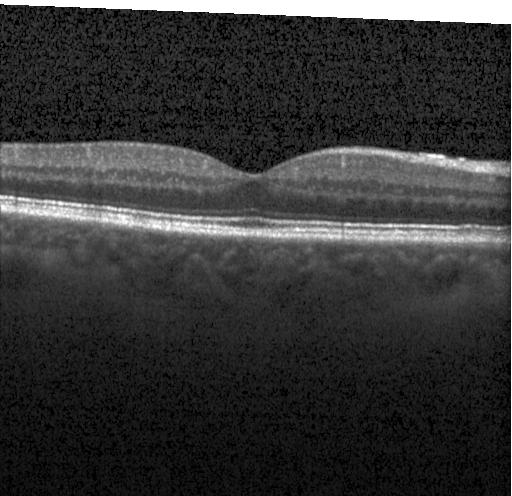

Heidelberg Spectralis · optical coherence tomography scan · centered on the fovea — Finding: no choroidal neovascularization, no diabetic macular edema, and no drusen.